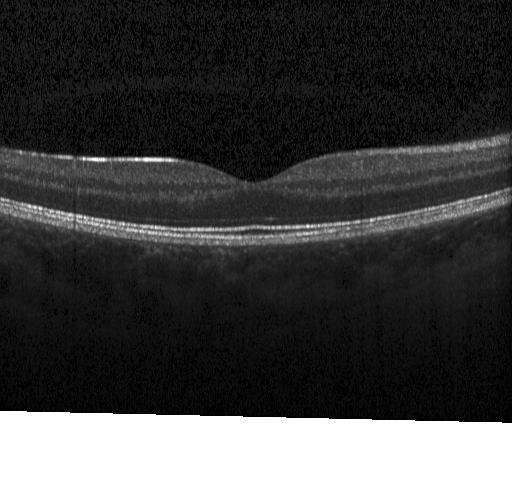

Finding: no choroidal neovascularization, diabetic macular edema, or drusen.